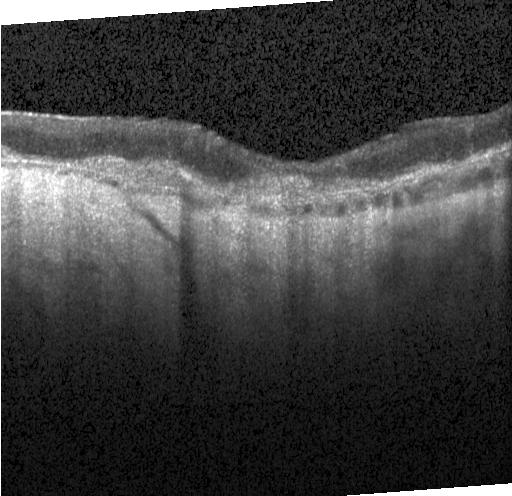 Spectral-domain OCT. Fovea-centered. Heidelberg Spectralis. Retinal OCT cross-section — Macular OCT: a choroidal neovascular membrane.